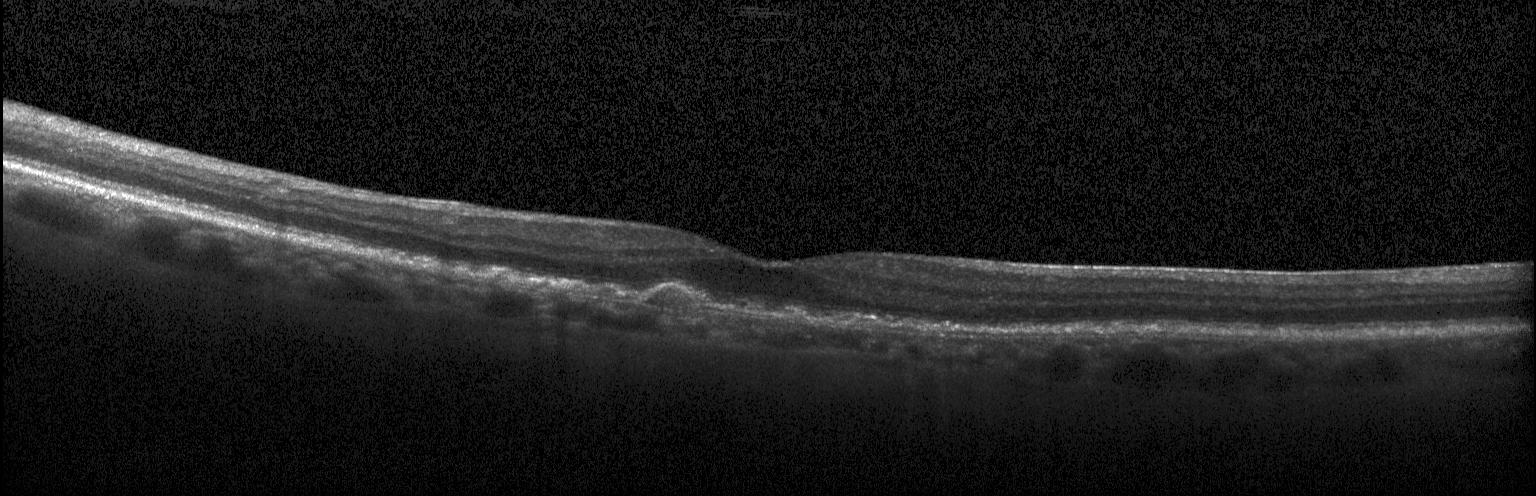

SD-OCT; through the macula; optical coherence tomography B-scan.
Diagnosis: multiple drusen.